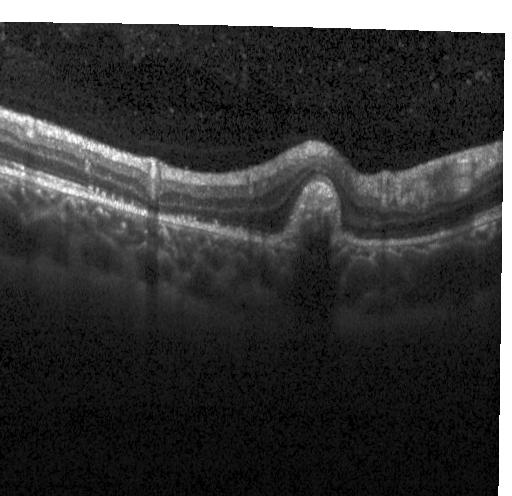

Spectral-domain optical coherence tomography. Retinal OCT B-scan
Diagnosis: a choroidal neovascular membrane.